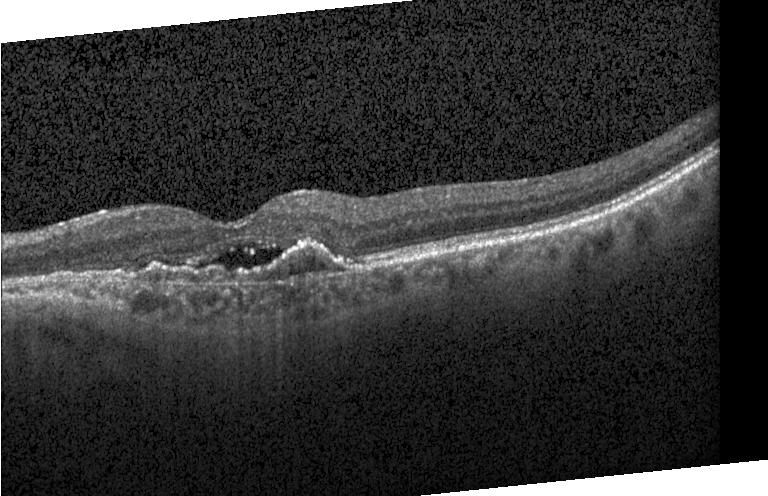
Optical coherence tomography scan. Acquired on a Heidelberg Spectralis. Through the macula. Spectral-domain optical coherence tomography.
Finding: a choroidal neovascular membrane.